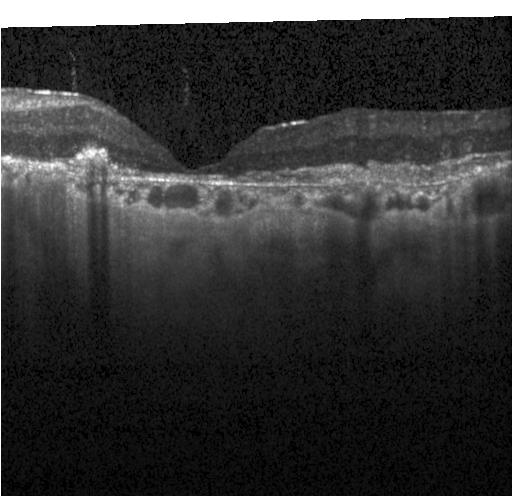

The scan shows a choroidal neovascular membrane.